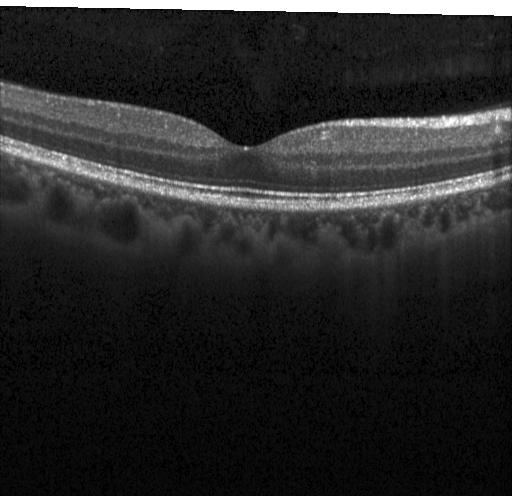

Optical coherence tomography scan — Macular OCT: no evidence of choroidal neovascularization, diabetic macular edema, or drusen.